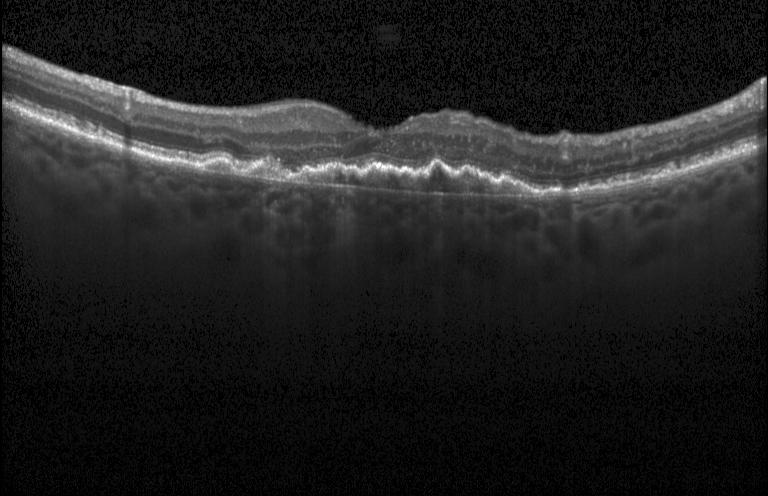

OCT scan showing CNV.